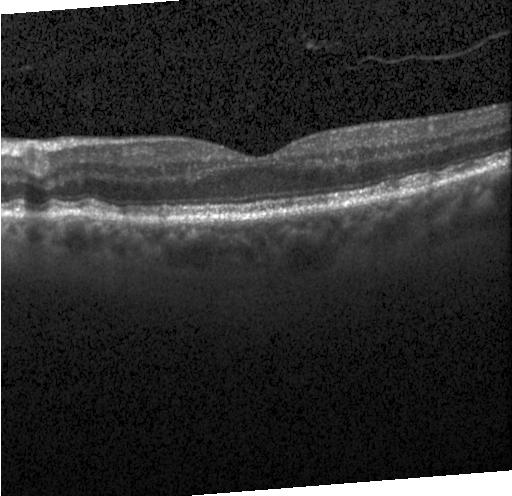
Spectral-domain optical coherence tomography; horizontal scan through the fovea; optical coherence tomography B-scan; Heidelberg Spectralis OCT system
Finding: drusen.